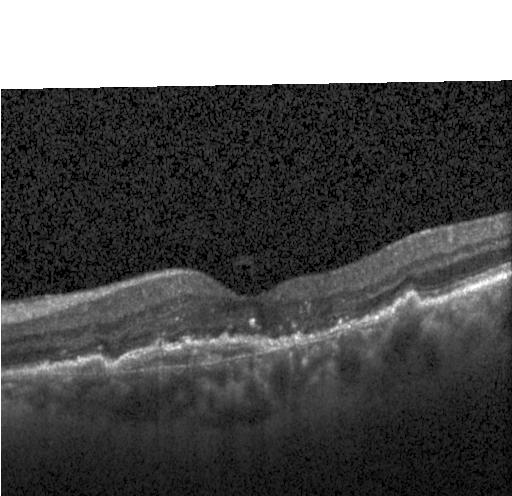

Impression: CNV.